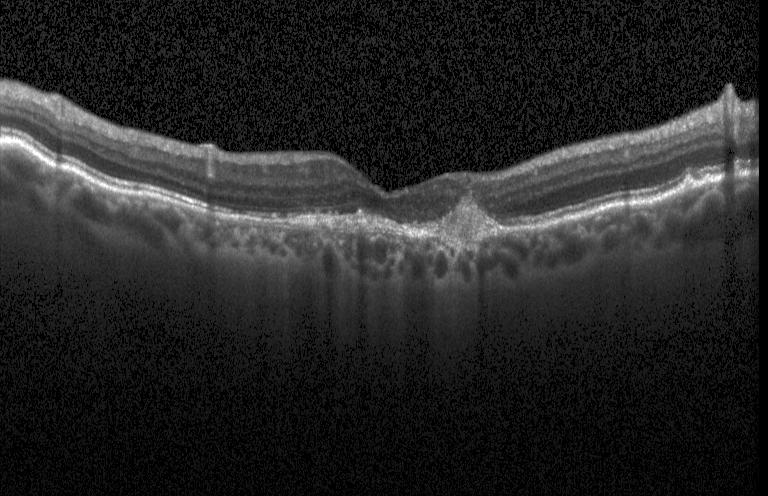 OCT B-scan; Heidelberg Spectralis.
This B-scan demonstrates a choroidal neovascular membrane.